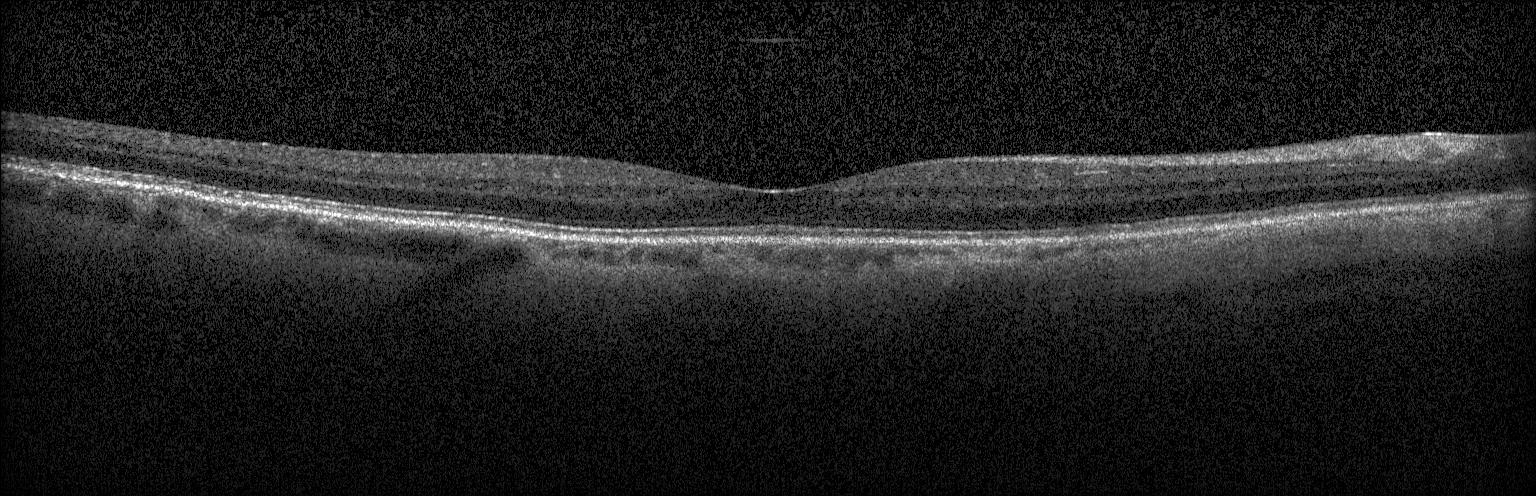 Retinal OCT B-scan. Diagnosis: no evidence of choroidal neovascularization, diabetic macular edema, or drusen.